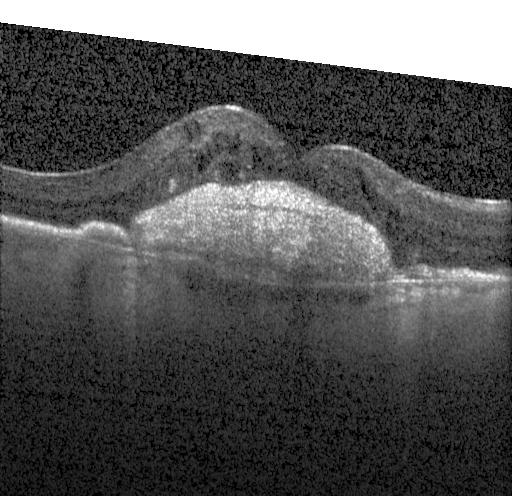

Optical coherence tomography B-scan, acquired on a Heidelberg Spectralis, spectral-domain OCT, fovea-centered.
Diagnosis: CNV.